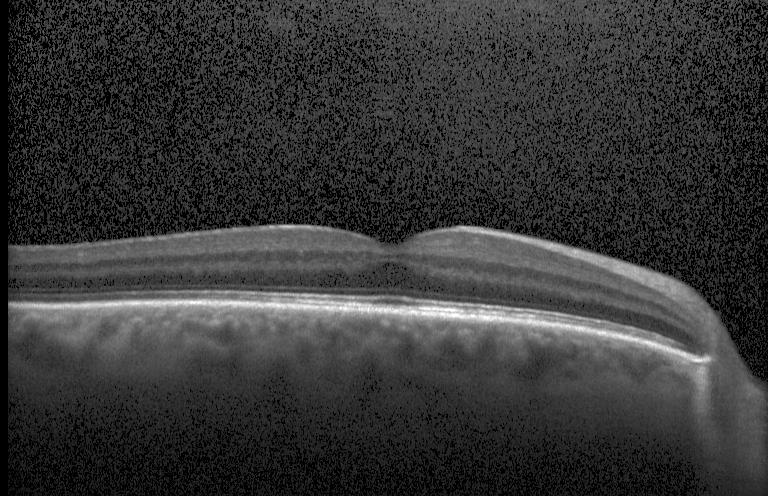
OCT B-scan. Impression: no choroidal neovascularization, no diabetic macular edema, and no drusen.